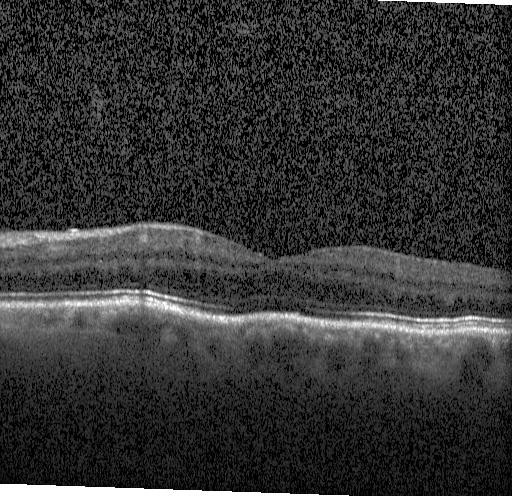

Diagnosis: no choroidal neovascularization, no diabetic macular edema, and no drusen.